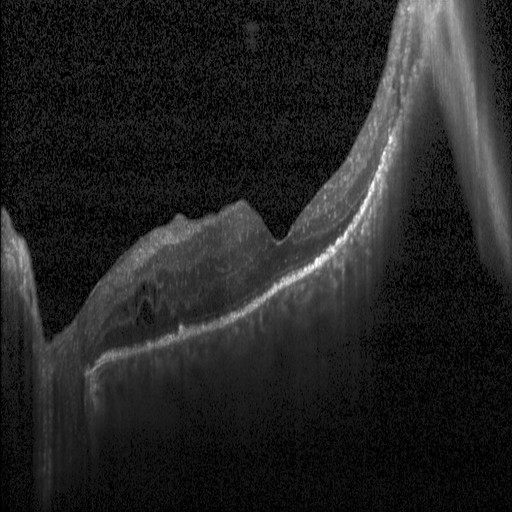

Retinal OCT cross-section · Heidelberg Spectralis OCT system · through the macula — Diabetic macular edema.